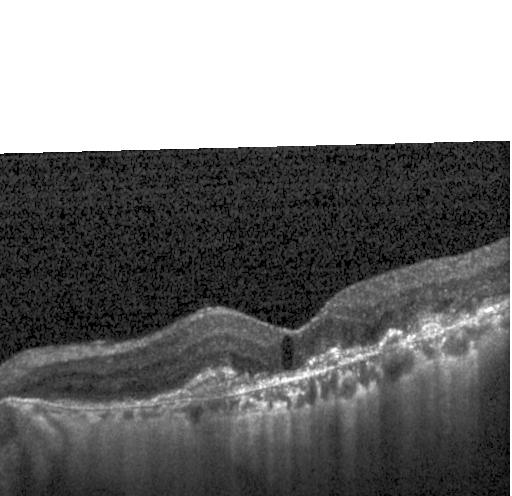 Assessment: CNV.